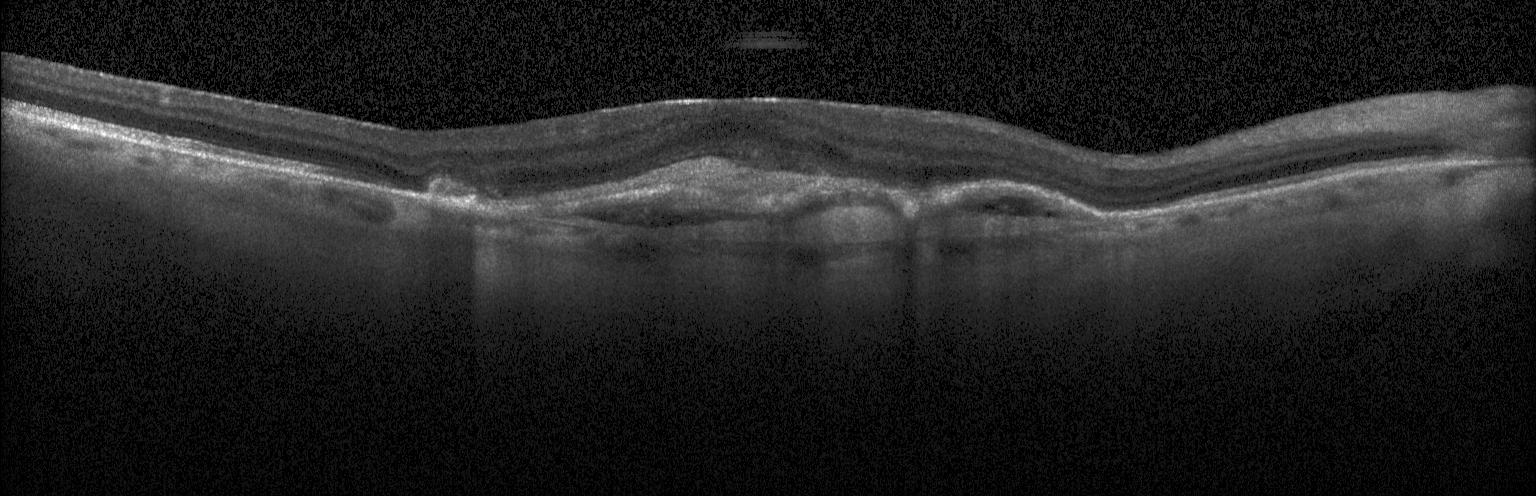 SD-OCT, retinal OCT cross-section.
Diagnosis: a choroidal neovascular membrane.